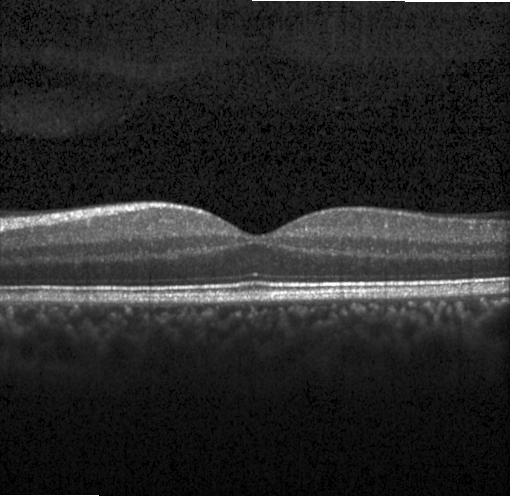
OCT B-scan showing no evidence of CNV, DME, or drusen.